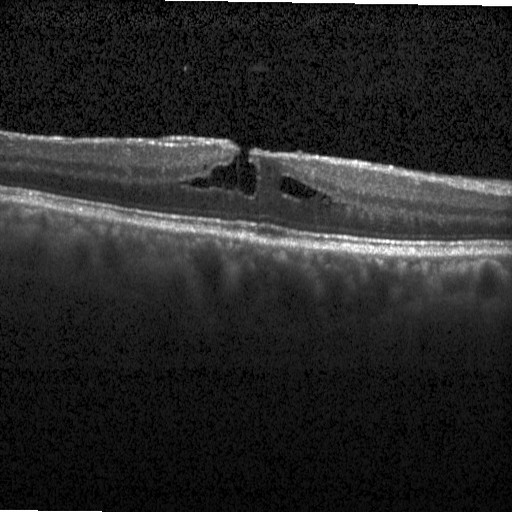 Horizontal scan through the fovea; optical coherence tomography scan; Heidelberg Spectralis; spectral-domain optical coherence tomography. The scan shows DME.